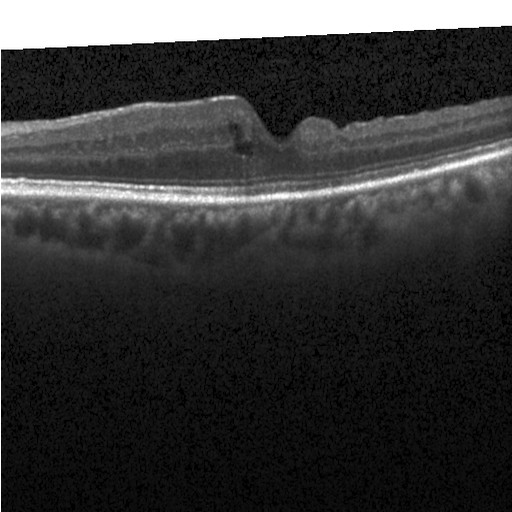

Dx: diabetic macular edema (DME).